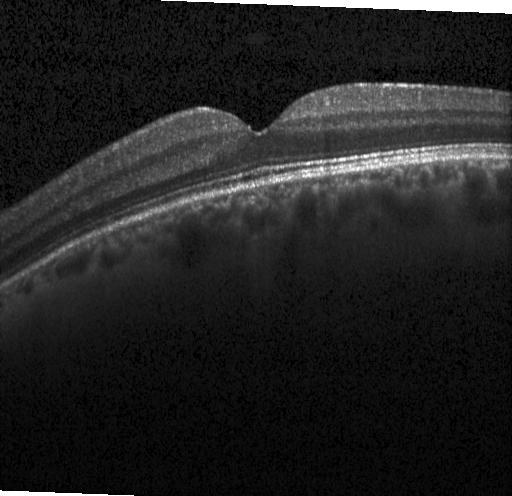
Horizontal scan through the fovea · optical coherence tomography scan · spectral-domain OCT
OCT finding: no choroidal neovascularization, no diabetic macular edema, and no drusen.